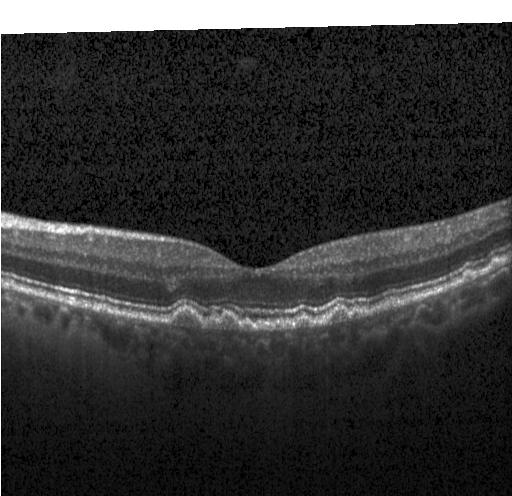 Optical coherence tomography B-scan, acquired on a Heidelberg Spectralis, spectral-domain OCT, through the macula — Finding: multiple drusen.